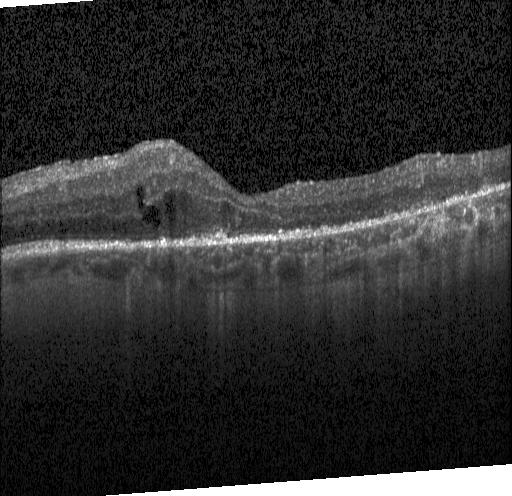 Spectral-domain OCT, instrument: Heidelberg Spectralis, optical coherence tomography B-scan, centered on the fovea. This B-scan demonstrates diabetic macular edema (DME).